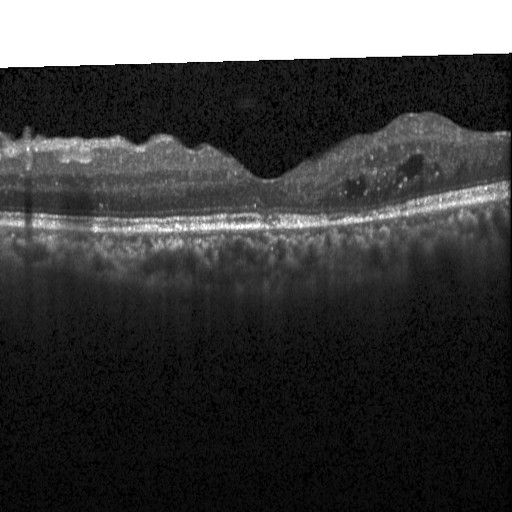
Horizontal scan through the fovea, instrument: Heidelberg Spectralis, OCT line scan, spectral-domain optical coherence tomography. Diagnosis: diabetic macular edema (DME).